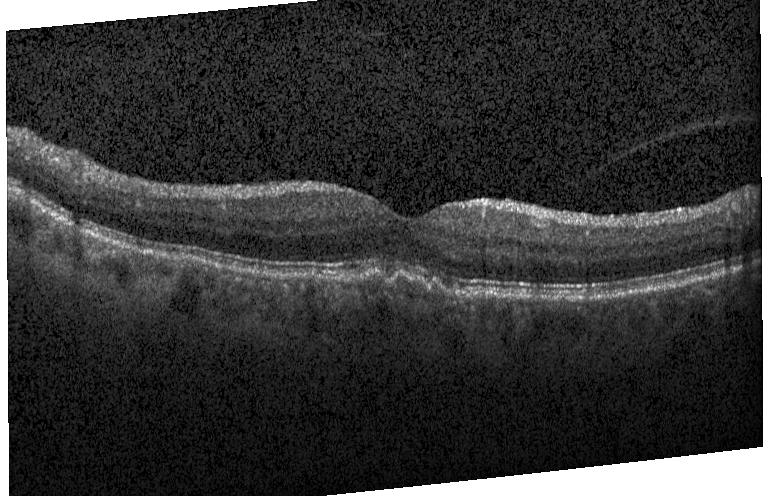

Impression: sub-RPE drusenoid deposits.